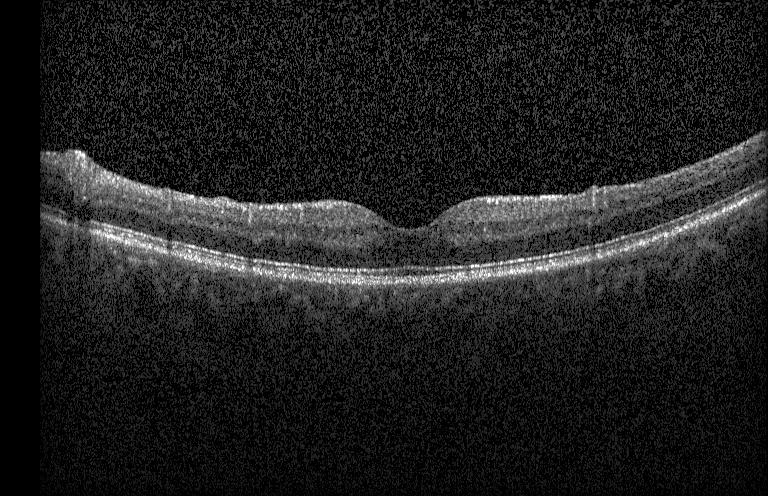

Finding: no choroidal neovascularization, no diabetic macular edema, and no drusen.